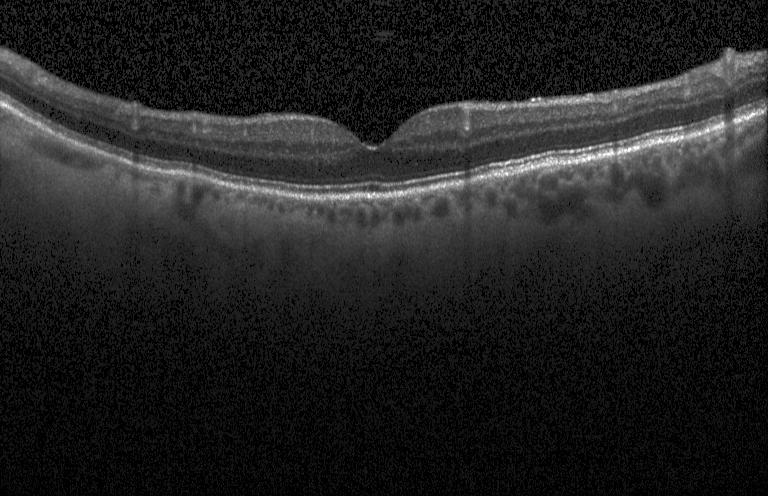

Spectral-domain OCT B-scan: no choroidal neovascularization, diabetic macular edema, or drusen.